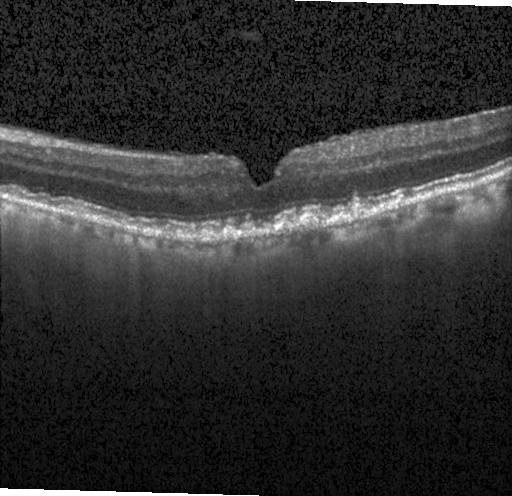

OCT B-scan — Assessment: sub-RPE drusenoid deposits.